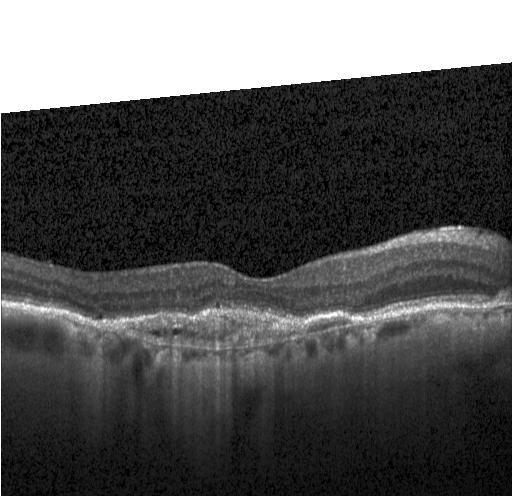

Through the macula · SD-OCT · optical coherence tomography B-scan — Macular OCT: choroidal neovascularization (CNV).